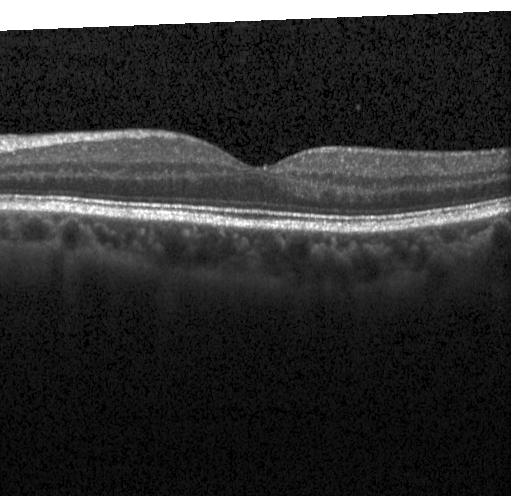
Finding: no CNV, DME, or drusen.